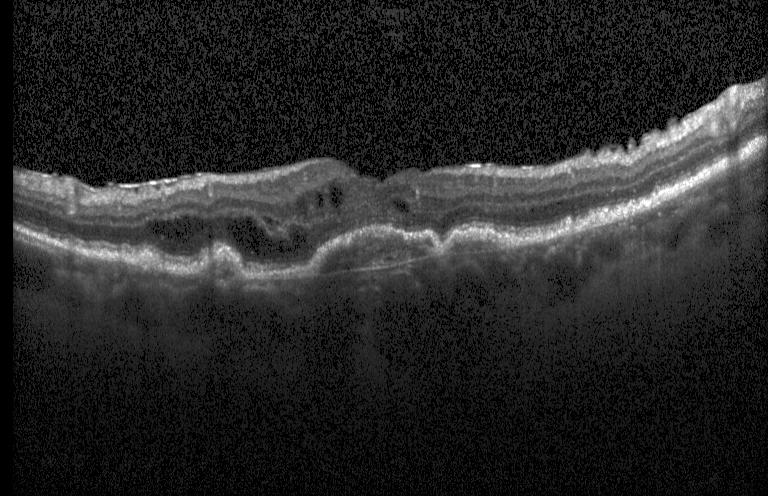 Impression: a choroidal neovascular membrane.